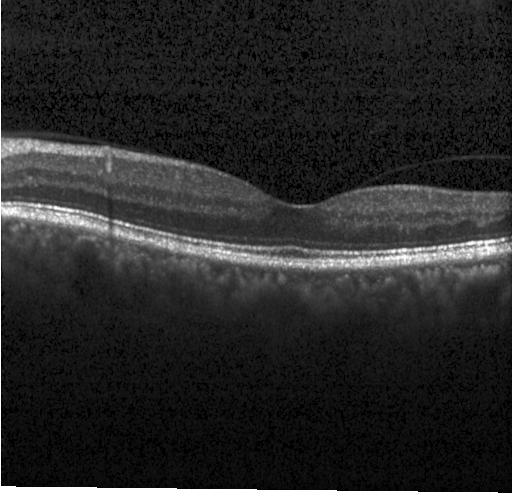

Retinal OCT cross-section. SD-OCT
Assessment: no evidence of choroidal neovascularization, diabetic macular edema, or drusen.